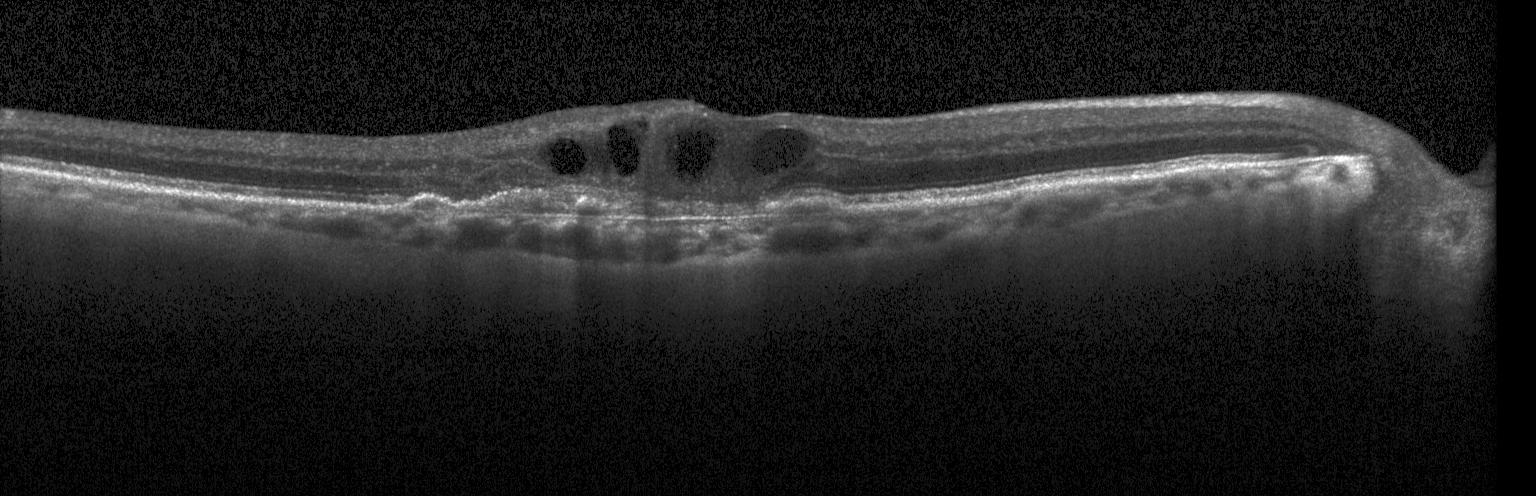
Heidelberg Spectralis. OCT B-scan. Centered on the fovea. This B-scan demonstrates choroidal neovascularization.